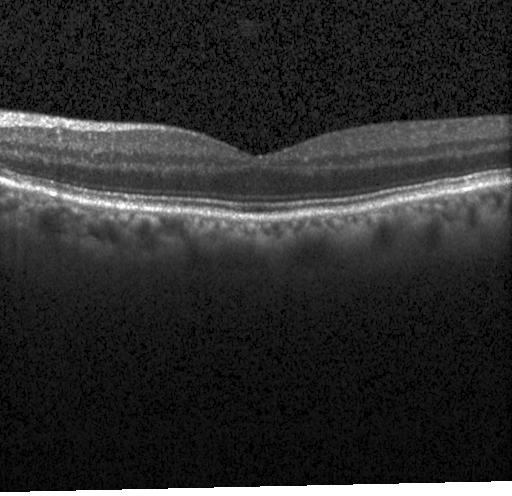 Dx: no evidence of choroidal neovascularization, diabetic macular edema, or drusen.